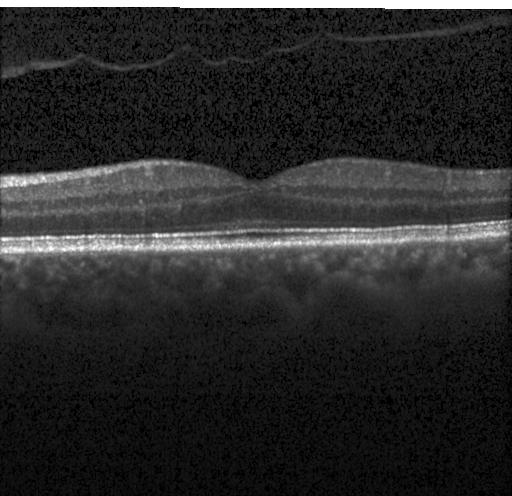
Spectral-domain optical coherence tomography · fovea-centered · retinal OCT cross-section — Finding: no CNV, DME, or drusen.